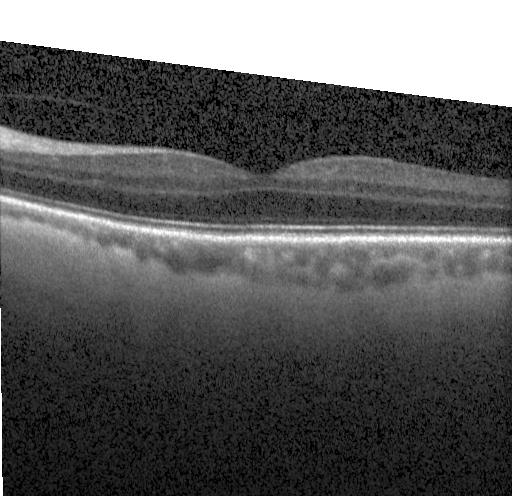
OCT finding: no CNV, no DME, and no drusen.